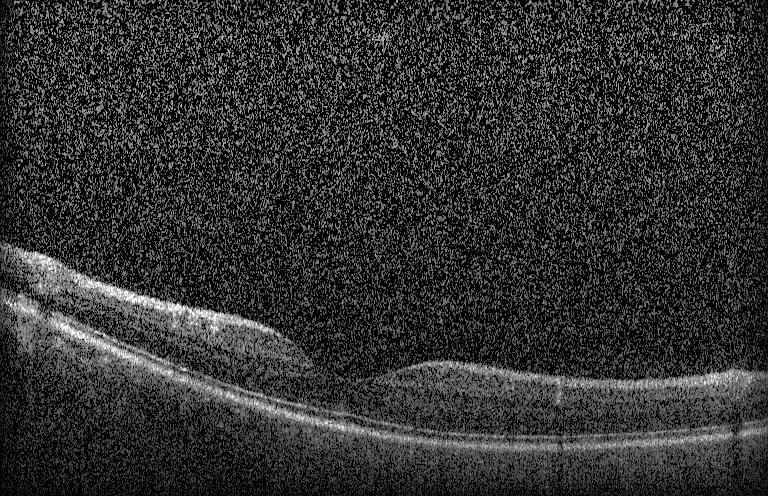 Retinal OCT cross-section · centered on the fovea · instrument: Heidelberg Spectralis.
Diagnosis: no evidence of choroidal neovascularization, diabetic macular edema, or drusen.